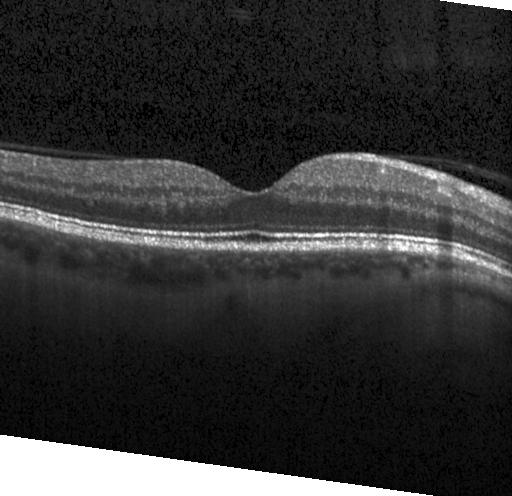
Horizontal scan through the fovea · optical coherence tomography scan.
The scan shows neither choroidal neovascularization, diabetic macular edema, nor drusen.